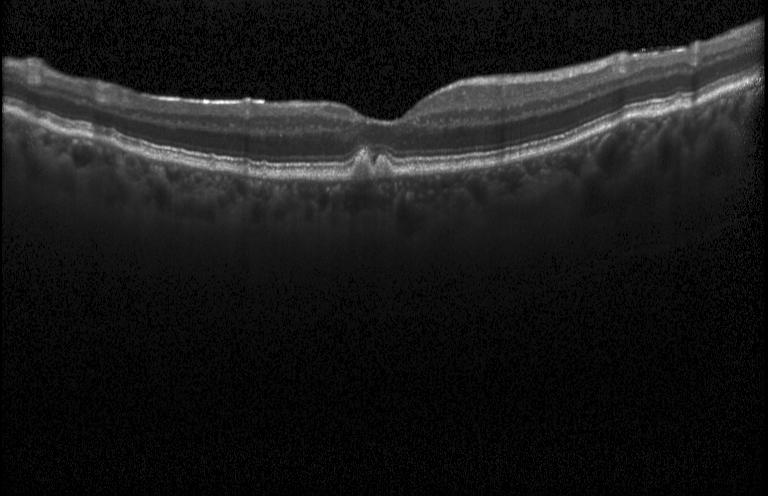
Spectral-domain OCT. OCT B-scan
Finding: sub-RPE drusenoid deposits.